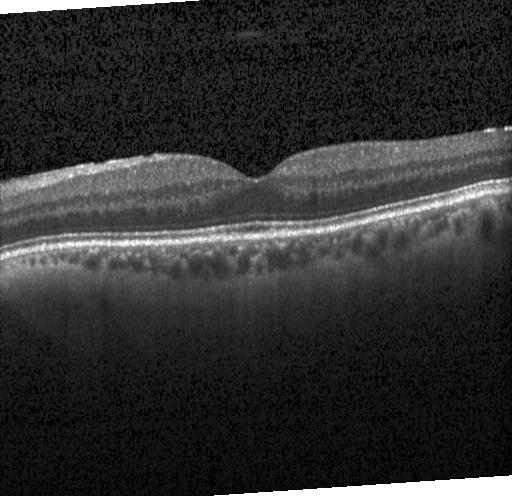

The scan shows no evidence of choroidal neovascularization, diabetic macular edema, or drusen.